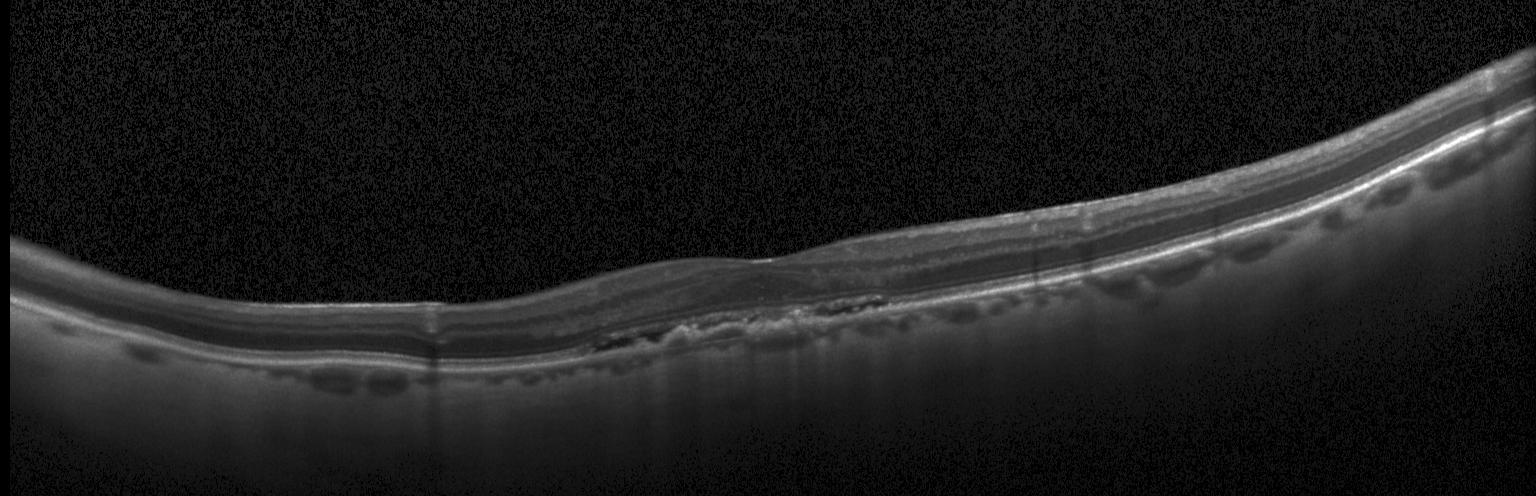 Diagnosis: choroidal neovascularization (CNV).